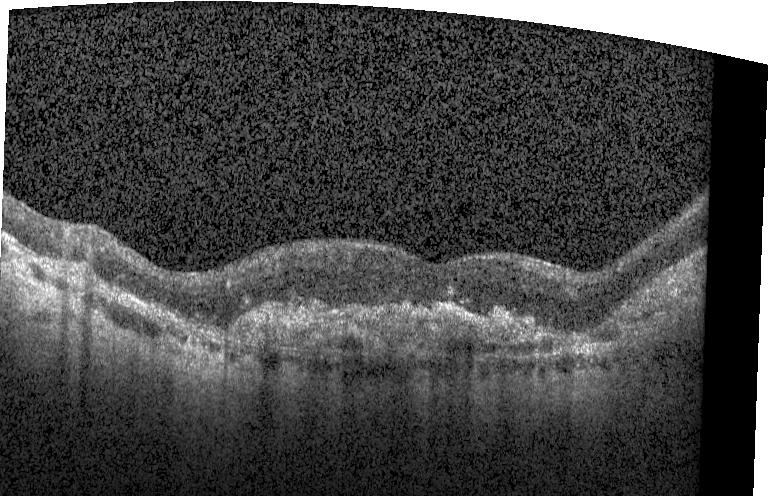
Macular scan; SD-OCT; optical coherence tomography B-scan; instrument: Heidelberg Spectralis — Finding: a choroidal neovascular membrane.